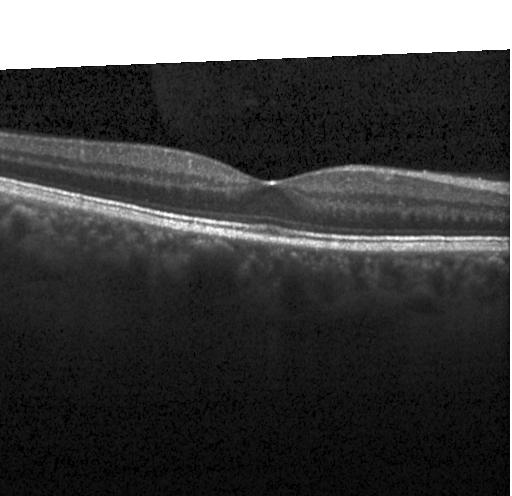 Finding: no choroidal neovascularization, diabetic macular edema, or drusen.